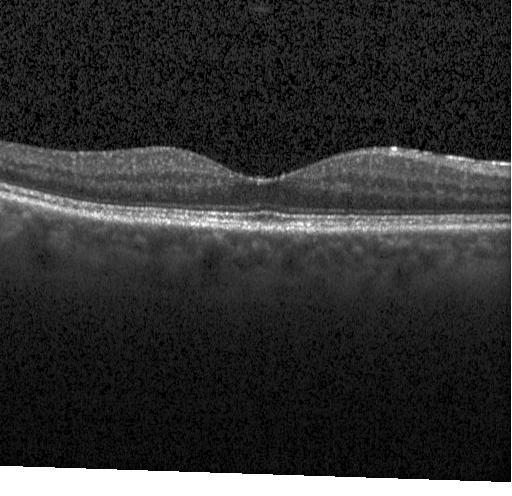
Retinal OCT cross-section — Impression: no choroidal neovascularization, no diabetic macular edema, and no drusen.